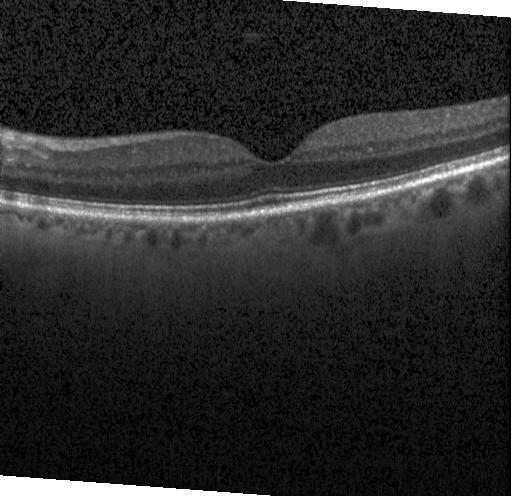
Impression: neither choroidal neovascularization, diabetic macular edema, nor drusen.